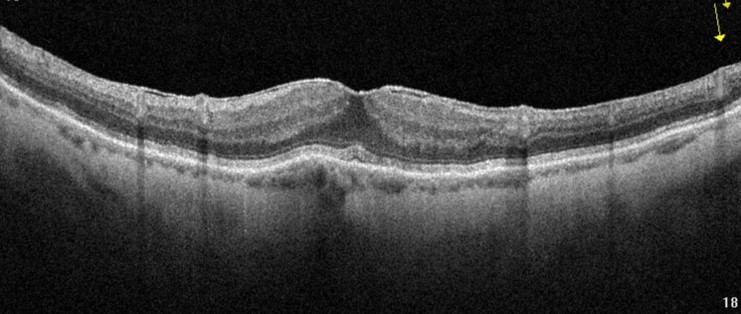 OCT scan showing age-related macular degeneration.